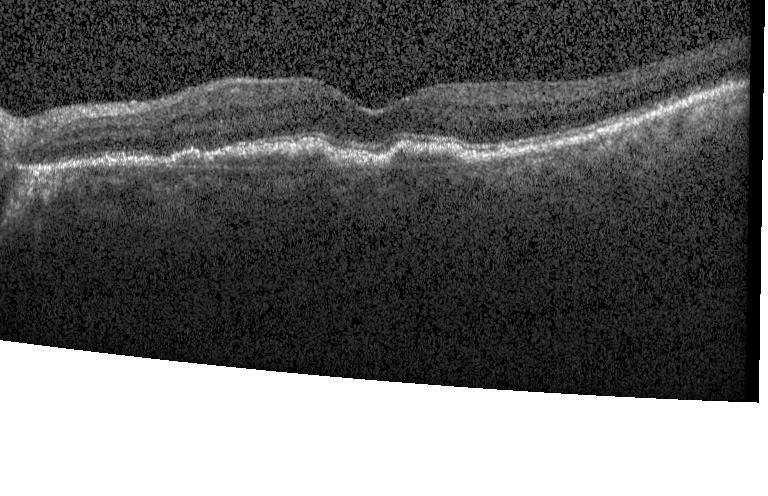

OCT B-scan showing CNV.